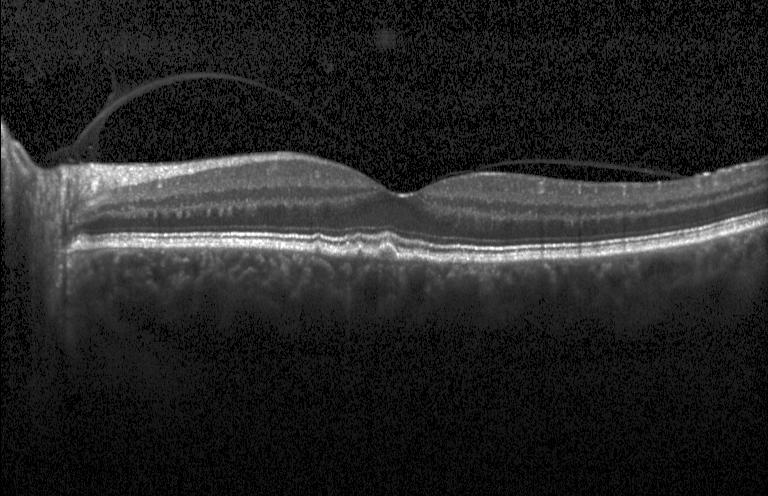

Spectral-domain OCT; retinal OCT B-scan; instrument: Heidelberg Spectralis — Macular OCT: multiple drusen.